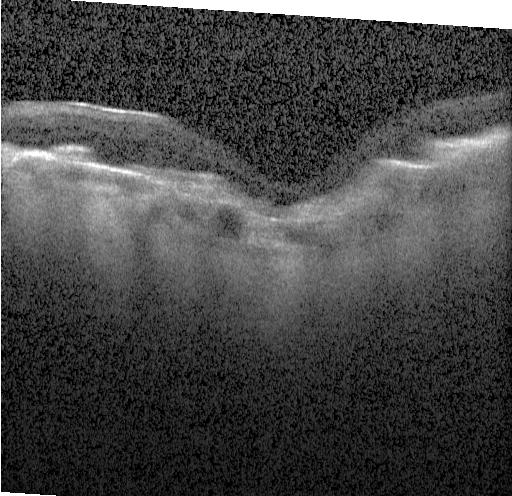 Through the macula; optical coherence tomography B-scan — Finding: choroidal neovascularization (CNV).